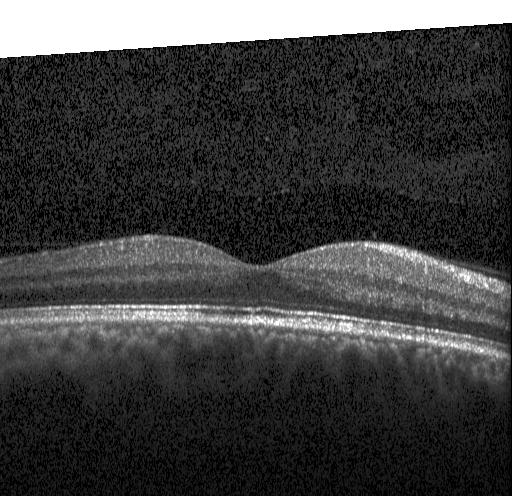

The scan shows no evidence of choroidal neovascularization, diabetic macular edema, or drusen.